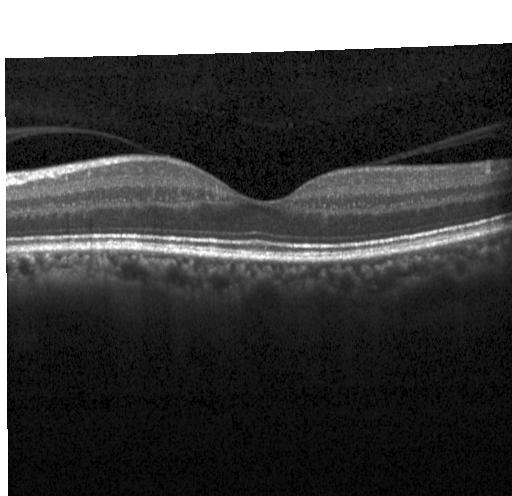

Dx: neither choroidal neovascularization, diabetic macular edema, nor drusen.